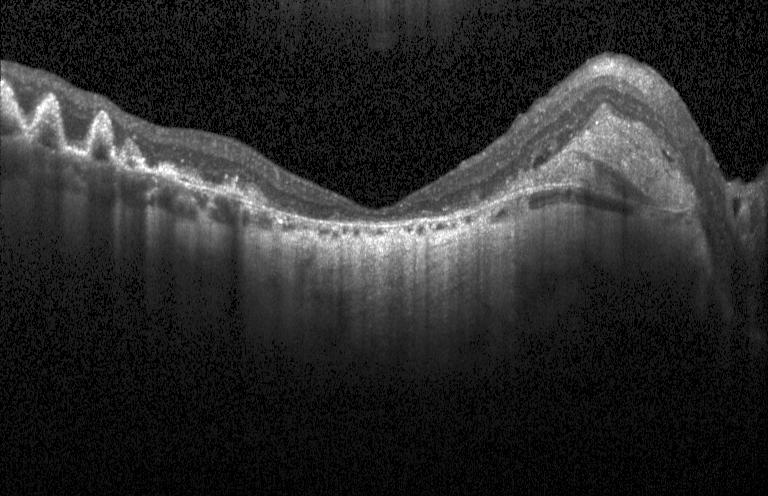
Impression: CNV.